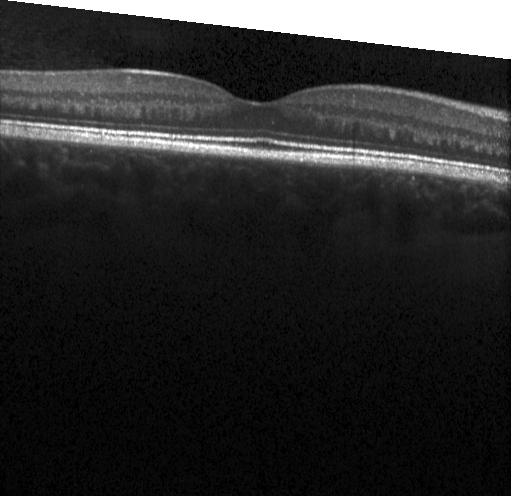 Spectral-domain OCT · retinal OCT B-scan — Impression: no choroidal neovascularization, no diabetic macular edema, and no drusen.